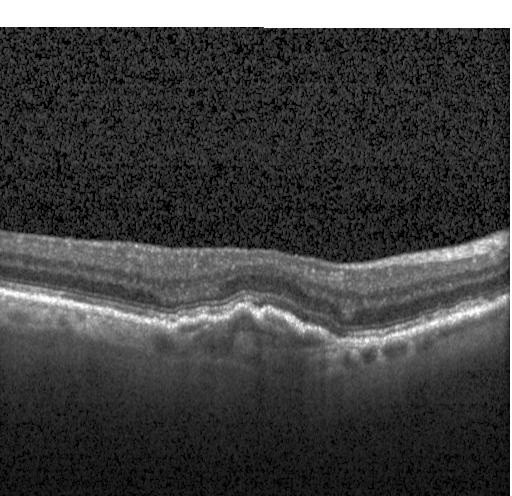
OCT line scan.
A choroidal neovascular membrane.